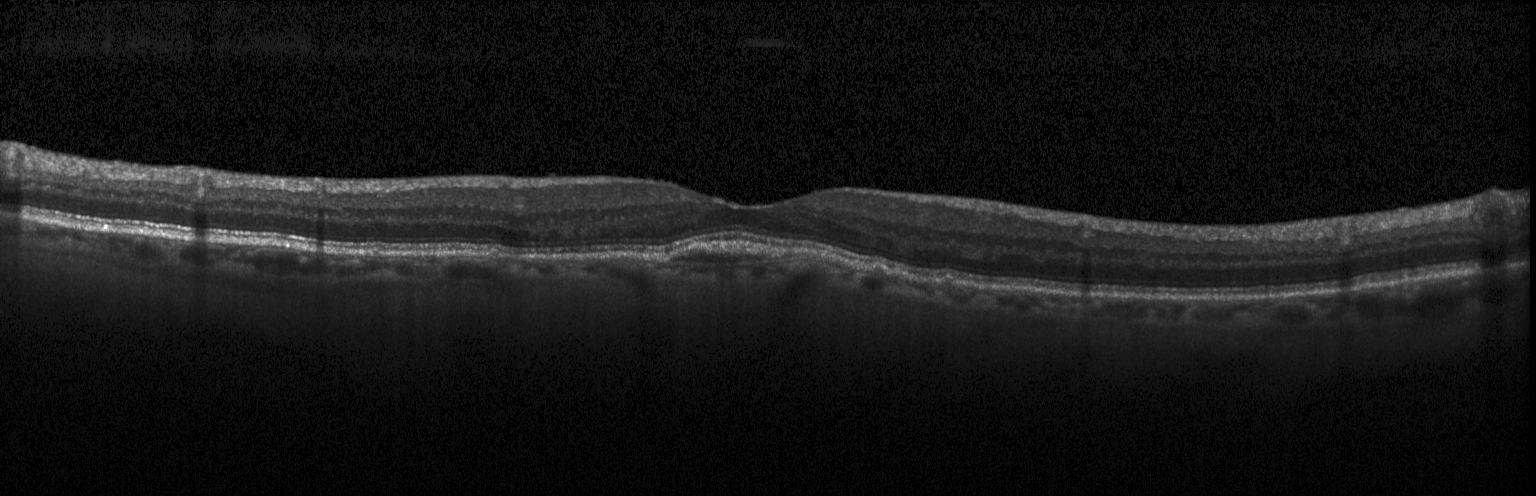
Dx: a choroidal neovascular membrane.